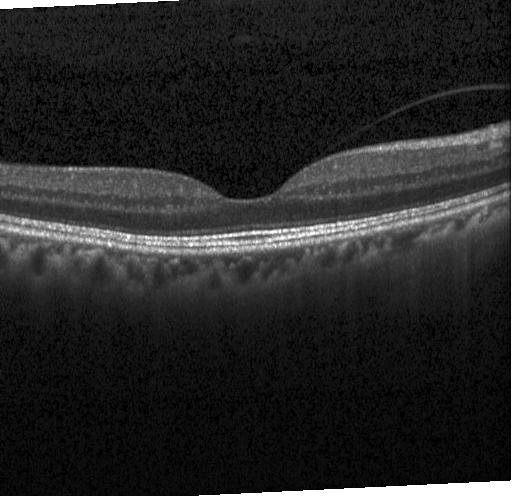

Diagnosis: no evidence of CNV, DME, or drusen.